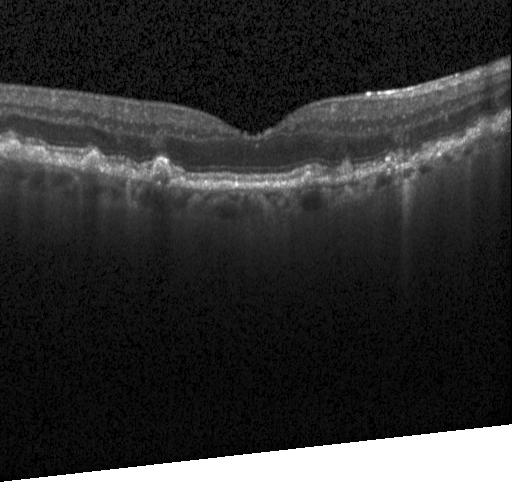 Finding: sub-RPE drusenoid deposits.